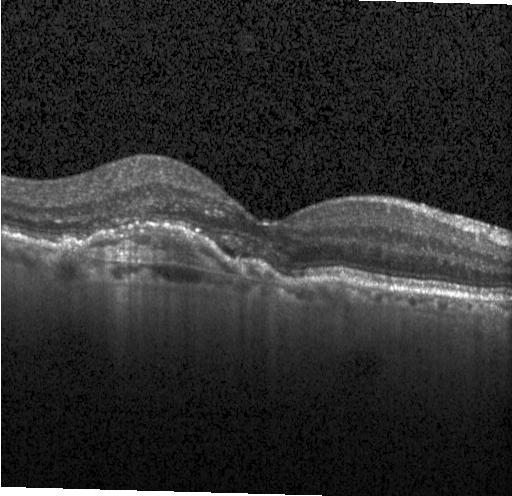 Diagnosis: a choroidal neovascular membrane.